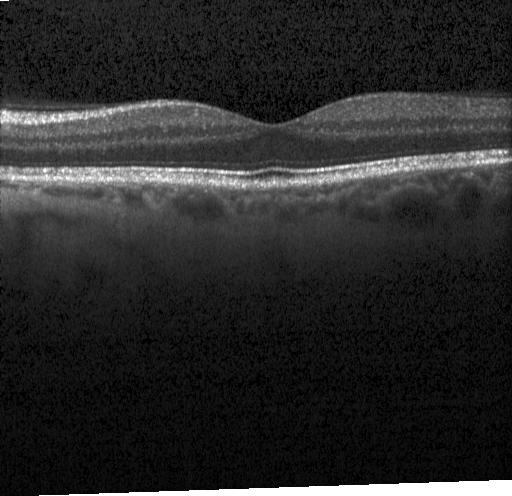
OCT B-scan — No evidence of choroidal neovascularization, diabetic macular edema, or drusen.